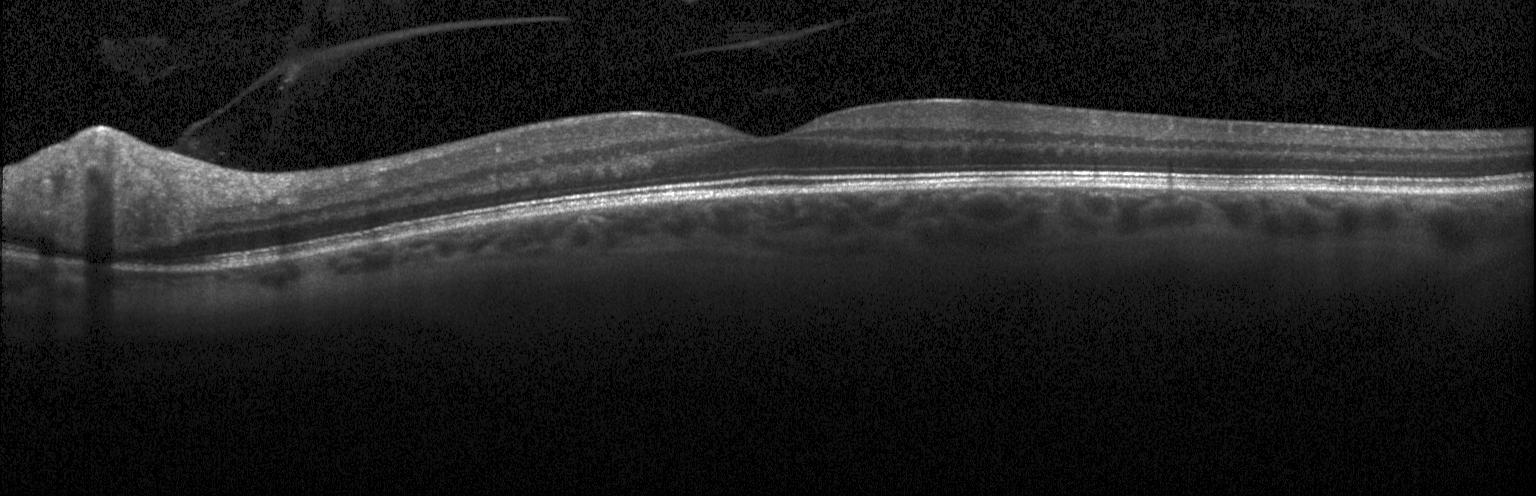
Optical coherence tomography scan. Spectral-domain OCT. Horizontal scan through the fovea. Heidelberg Spectralis. Assessment: no CNV, DME, or drusen.